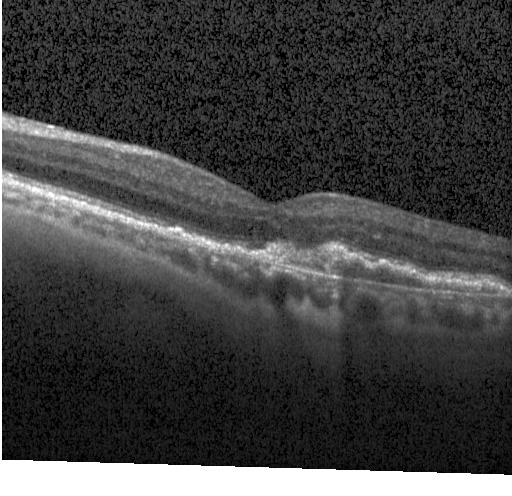
Retinal OCT cross-section showing a choroidal neovascular membrane.